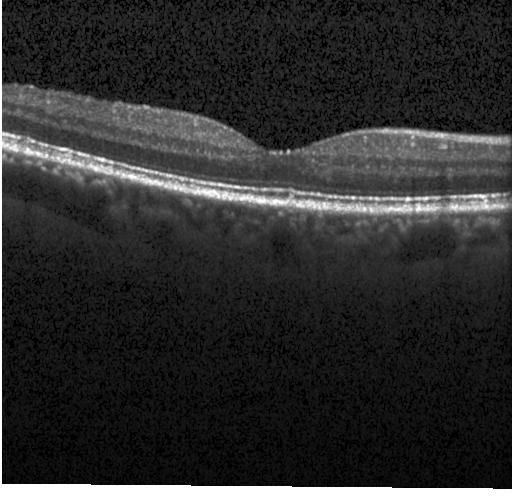
Optical coherence tomography B-scan — Macular OCT: no choroidal neovascularization, no diabetic macular edema, and no drusen.